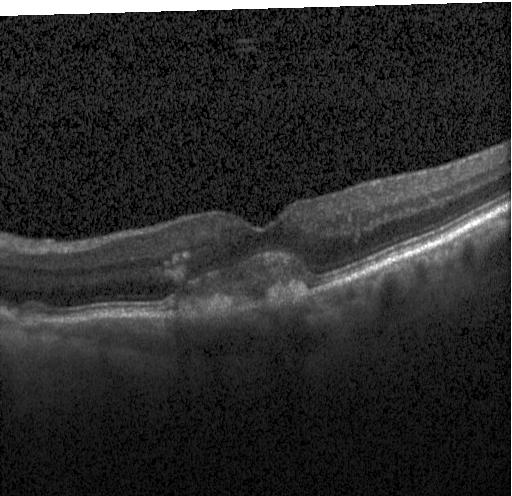
OCT line scan.
This B-scan demonstrates CNV.